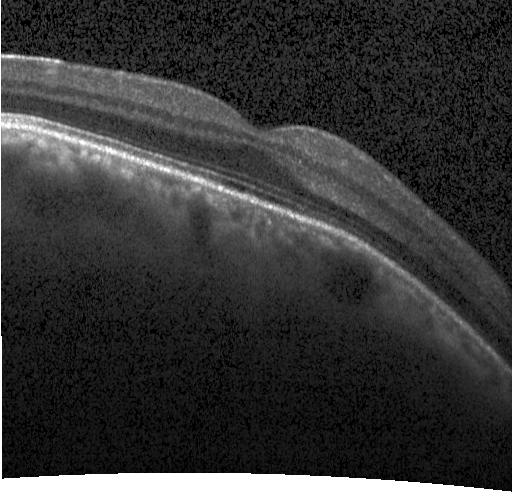 OCT line scan. Macular OCT: no evidence of choroidal neovascularization, diabetic macular edema, or drusen.